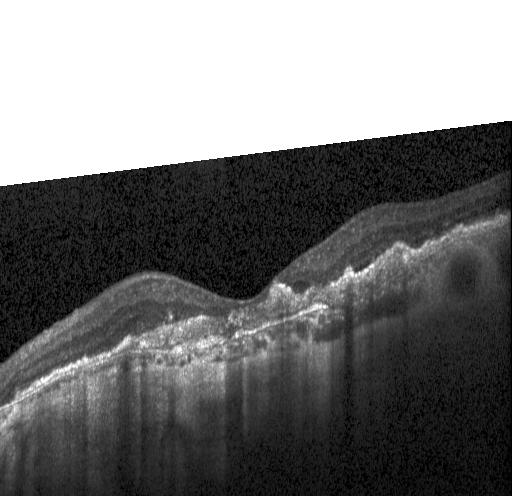

Impression: choroidal neovascularization.